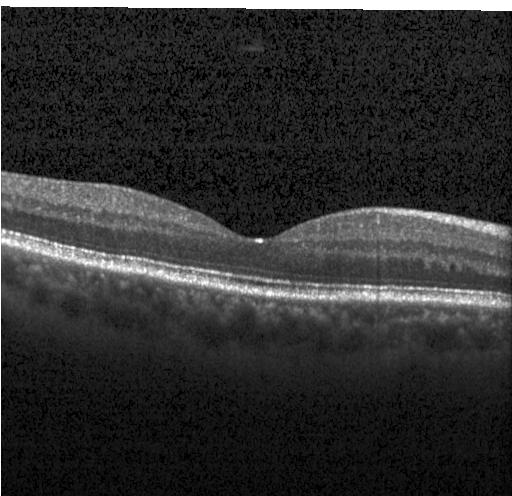 Diagnosis: no evidence of choroidal neovascularization, diabetic macular edema, or drusen.